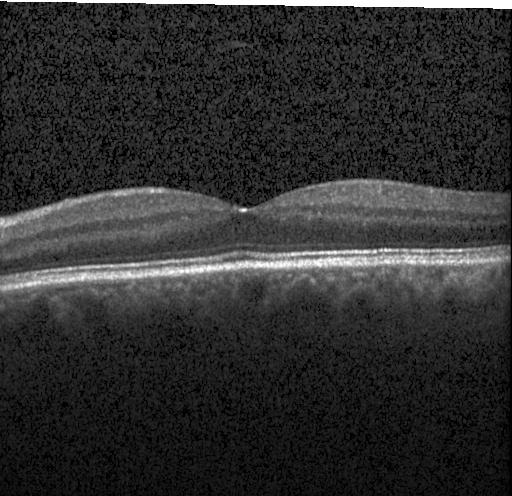
Instrument: Heidelberg Spectralis · spectral-domain OCT · optical coherence tomography scan · centered on the fovea. Diagnosis: neither CNV, DME, nor drusen.